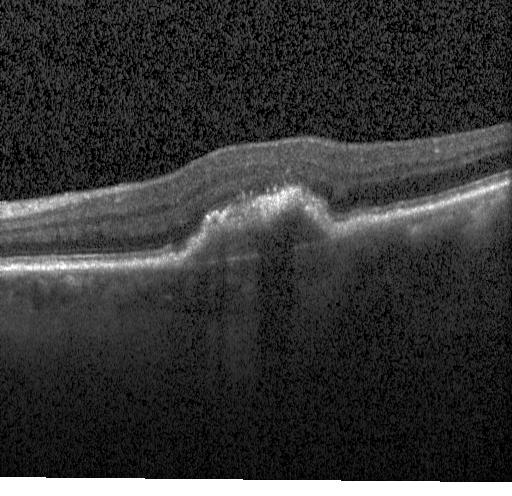
Retinal OCT cross-section, through the macula, SD-OCT, acquired on a Heidelberg Spectralis. Choroidal neovascularization (CNV).